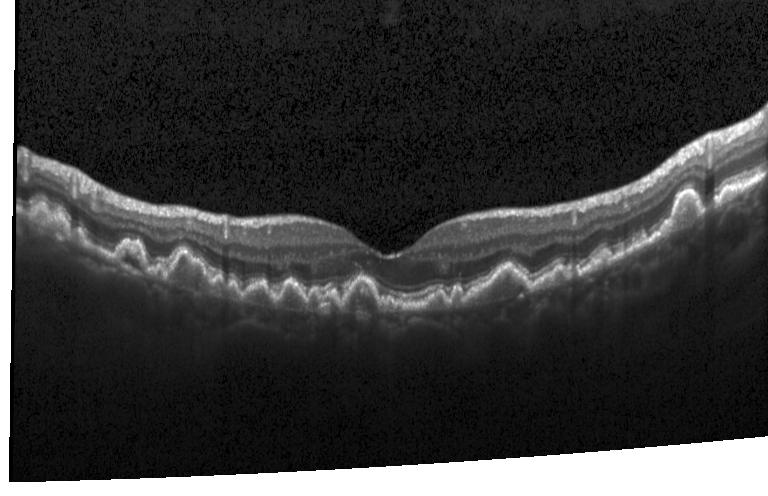 Optical coherence tomography B-scan, spectral-domain OCT
OCT finding: choroidal neovascularization.